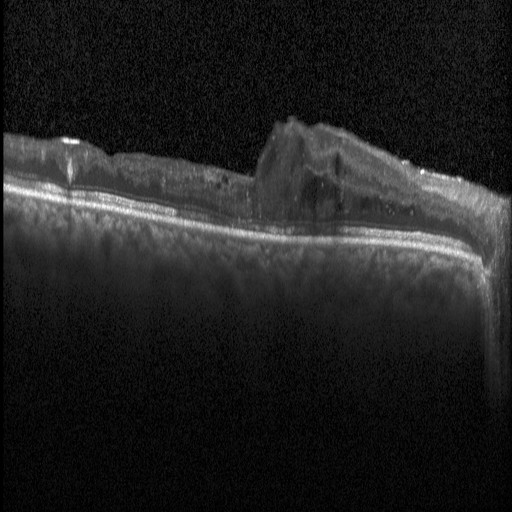 OCT B-scan; Heidelberg Spectralis; SD-OCT
OCT finding: DME.